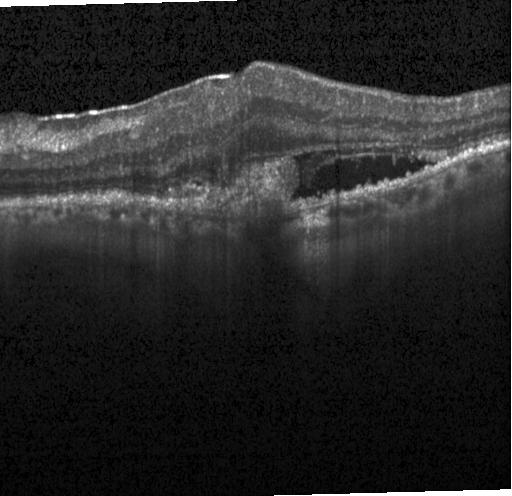

SD-OCT; instrument: Heidelberg Spectralis; through the macula; retinal OCT cross-section. Impression: a choroidal neovascular membrane.